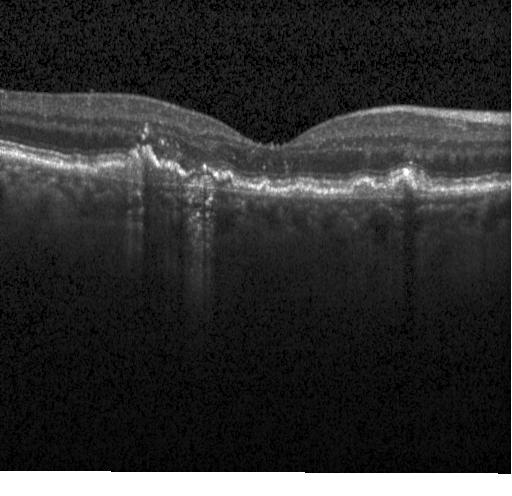
Diagnosis: a choroidal neovascular membrane.